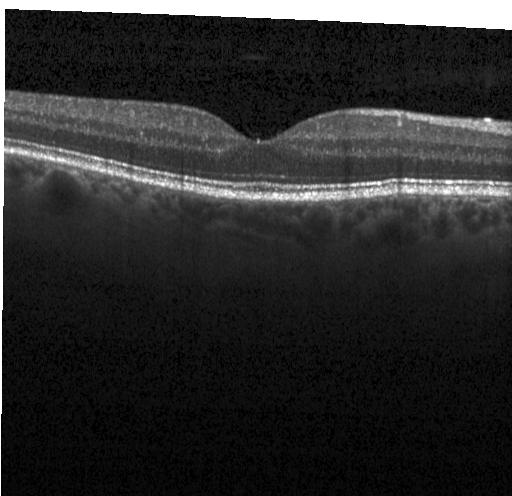
Retinal OCT cross-section showing neither choroidal neovascularization, diabetic macular edema, nor drusen.